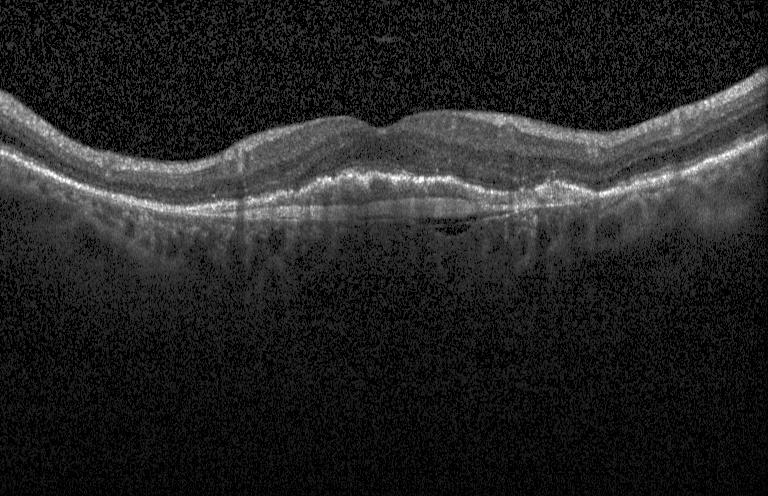
Retinal OCT cross-section · spectral-domain OCT — OCT finding: choroidal neovascularization (CNV).